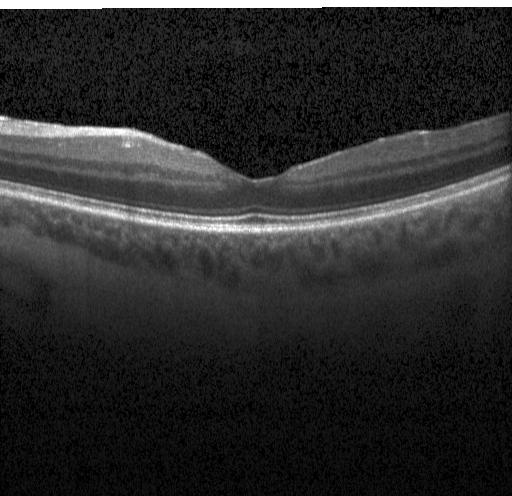

Retinal OCT cross-section, acquired on a Heidelberg Spectralis, SD-OCT, horizontal scan through the fovea — Assessment: no choroidal neovascularization, diabetic macular edema, or drusen.